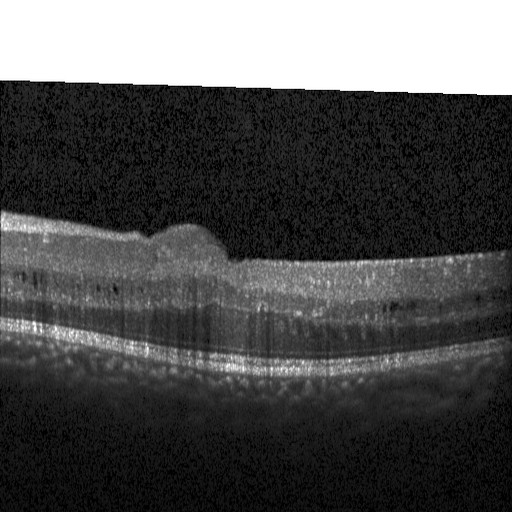
Optical coherence tomography scan, horizontal scan through the fovea, instrument: Heidelberg Spectralis — Finding: DME.